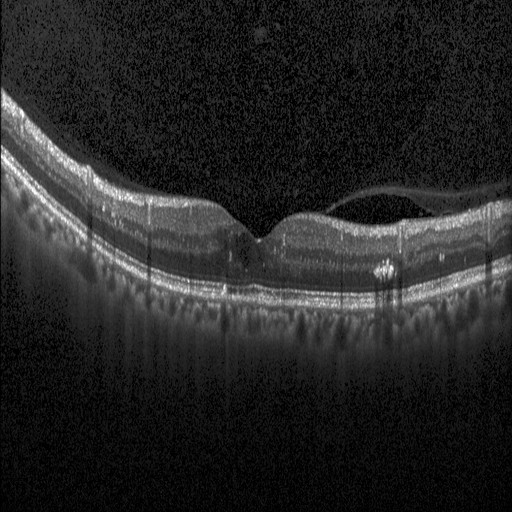 OCT scan showing diabetic macular edema (DME).